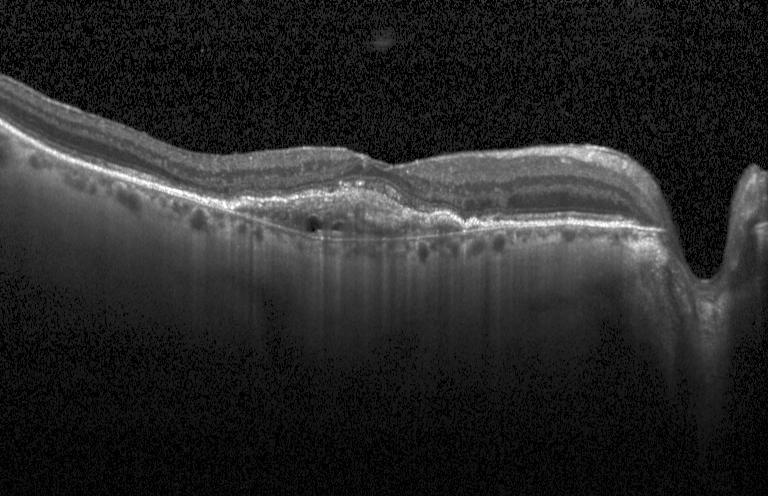

Macular OCT demonstrating a choroidal neovascular membrane.